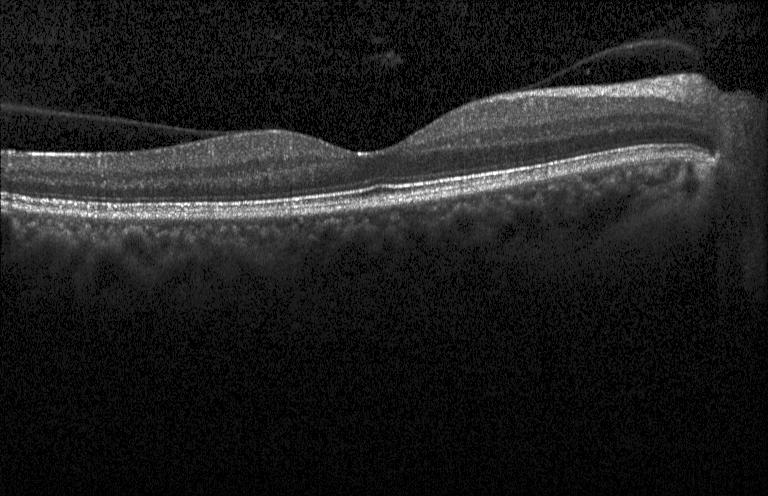 OCT B-scan. Acquired on a Heidelberg Spectralis. Macular scan
The scan shows no CNV, no DME, and no drusen.